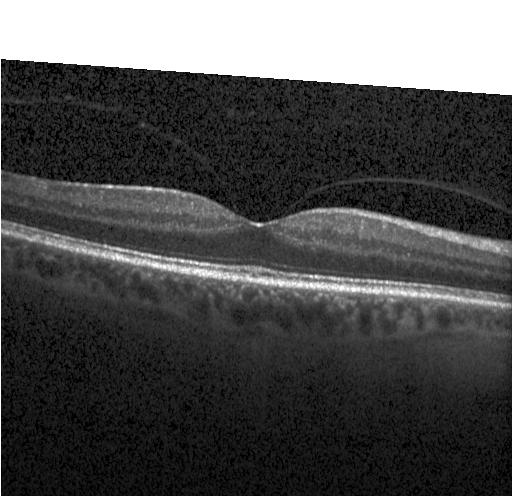 Centered on the fovea; instrument: Heidelberg Spectralis; OCT line scan — Diagnosis: no evidence of choroidal neovascularization, diabetic macular edema, or drusen.